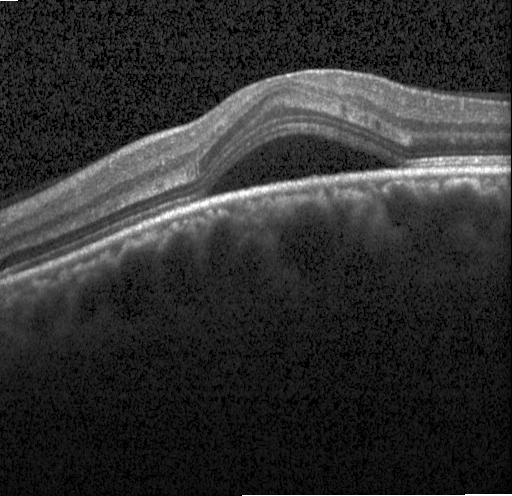
Optical coherence tomography B-scan.
Finding: a choroidal neovascular membrane.